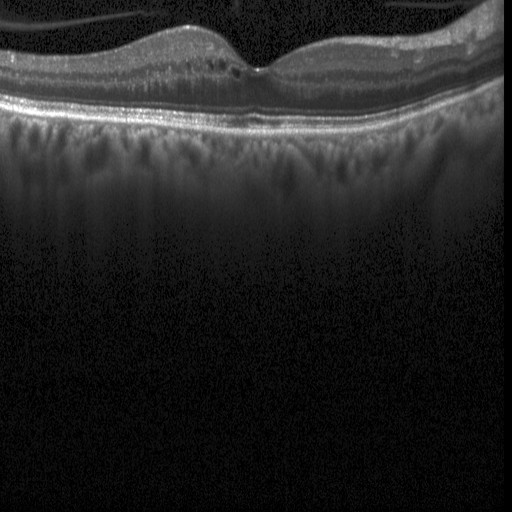 Heidelberg Spectralis OCT system; SD-OCT; optical coherence tomography B-scan.
Dx: diabetic macular edema (DME).